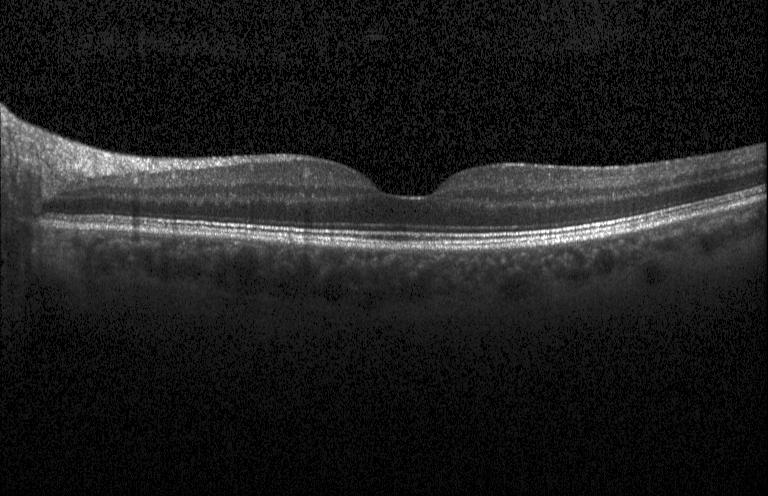

OCT scan showing no CNV, DME, or drusen.